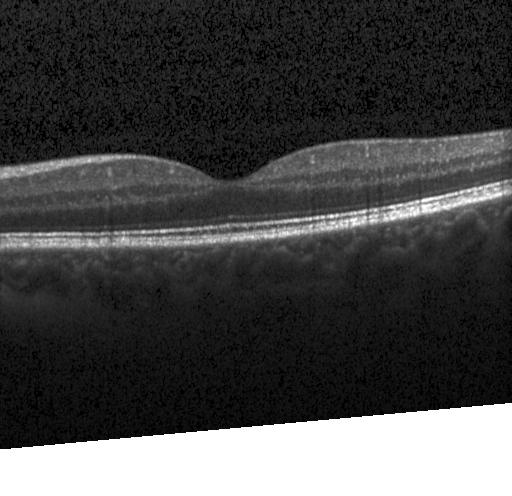 Diagnosis: neither CNV, DME, nor drusen.